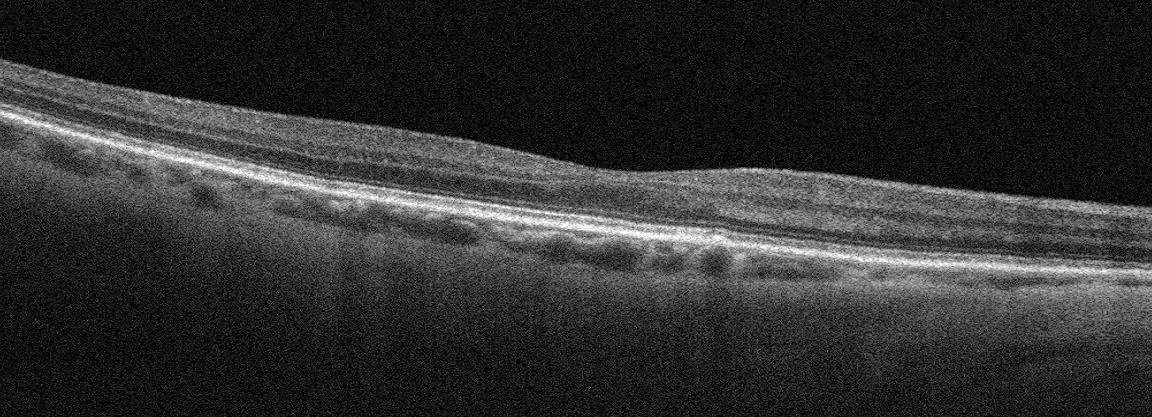
OCT B-scan — This B-scan demonstrates age-related macular degeneration (AMD).